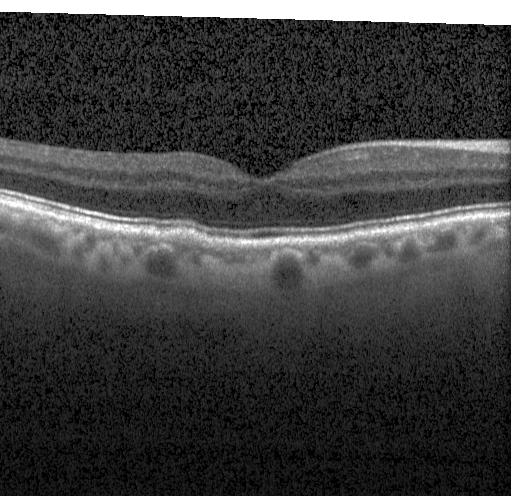

Sub-RPE drusenoid deposits.